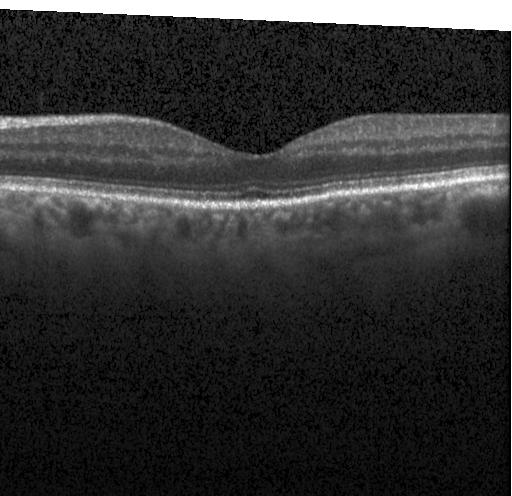
Spectral-domain OCT · retinal OCT cross-section — This B-scan demonstrates no evidence of choroidal neovascularization, diabetic macular edema, or drusen.